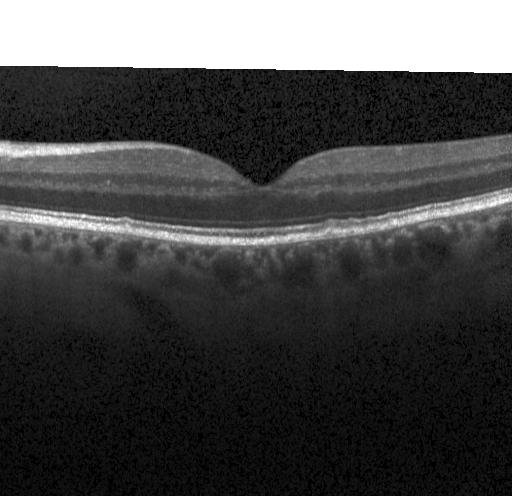
Macular scan · acquired on a Heidelberg Spectralis · optical coherence tomography B-scan. Finding: drusen.